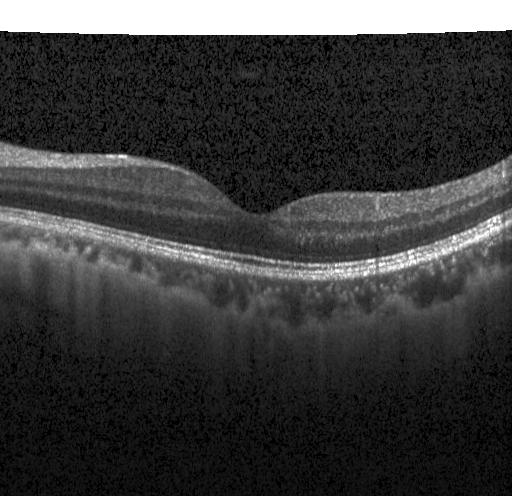 Acquired on a Heidelberg Spectralis; optical coherence tomography scan; SD-OCT; macular scan — Diagnosis: no choroidal neovascularization, diabetic macular edema, or drusen.